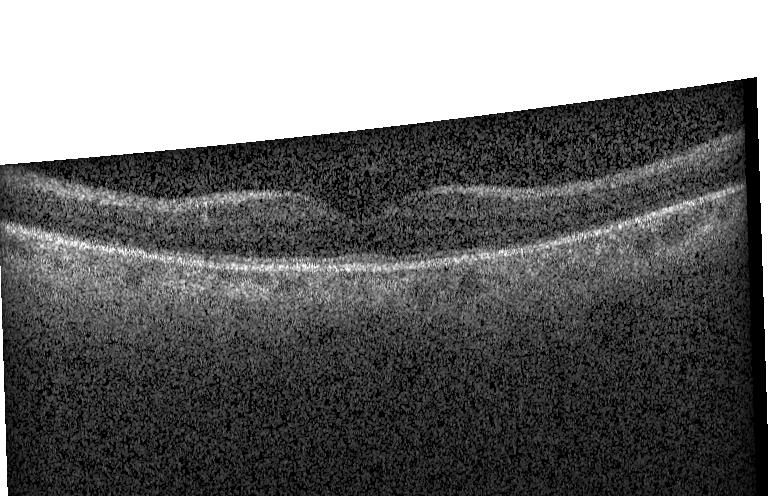 Retinal OCT B-scan
This B-scan demonstrates no choroidal neovascularization, diabetic macular edema, or drusen.